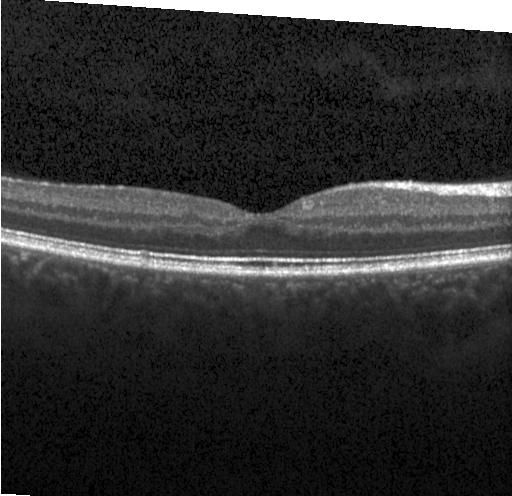
SD-OCT, OCT B-scan, Heidelberg Spectralis, through the macula. Dx: no choroidal neovascularization, diabetic macular edema, or drusen.